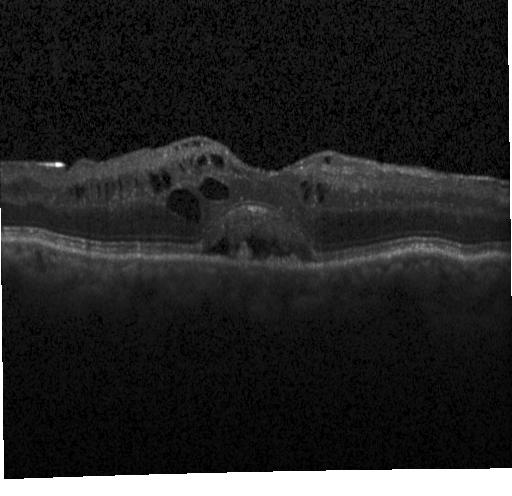
Heidelberg Spectralis, OCT line scan, centered on the fovea, spectral-domain optical coherence tomography. OCT finding: DME.